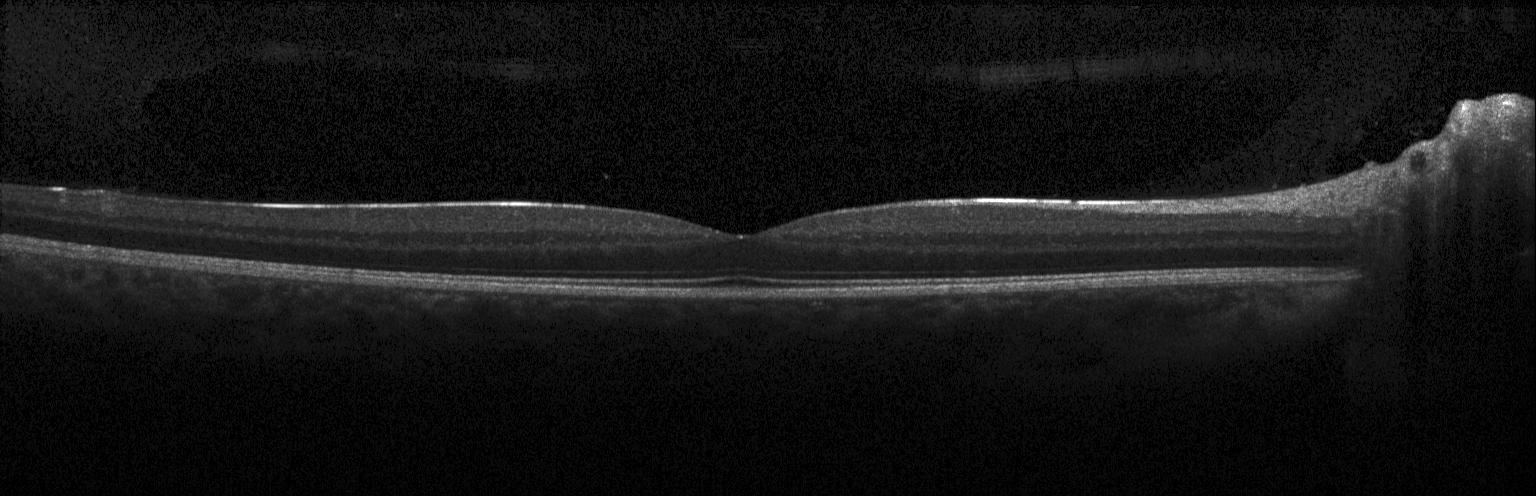 Finding: no choroidal neovascularization, diabetic macular edema, or drusen.